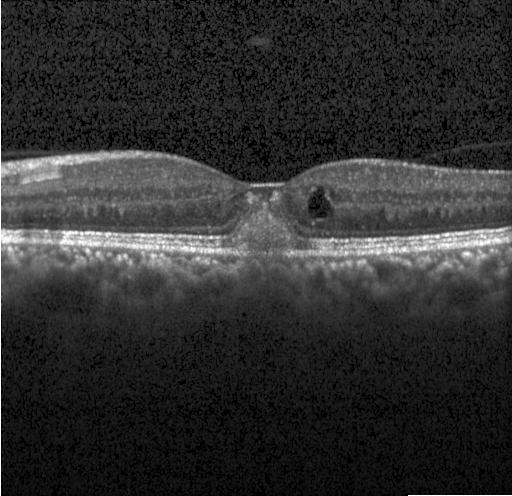

Acquired on a Heidelberg Spectralis · OCT line scan · horizontal scan through the fovea · SD-OCT — Choroidal neovascularization (CNV).